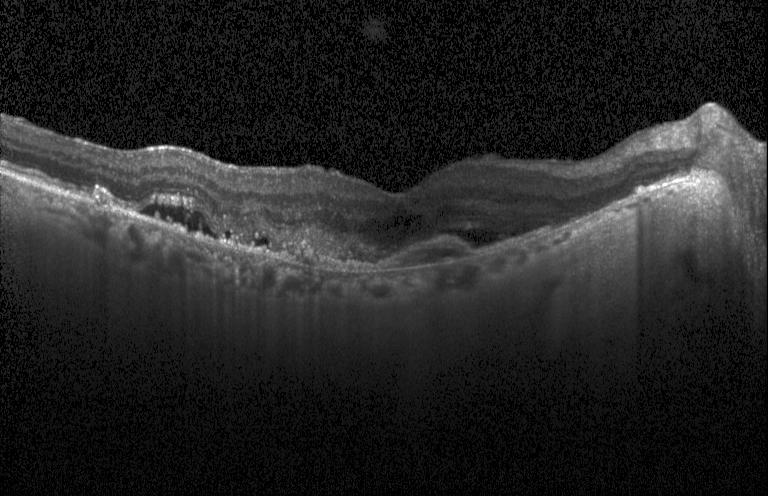 Macular OCT: CNV.